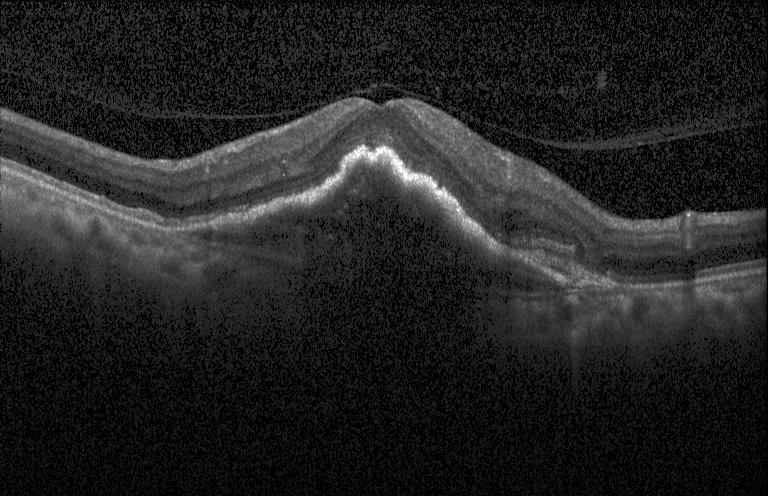 OCT B-scan showing CNV.